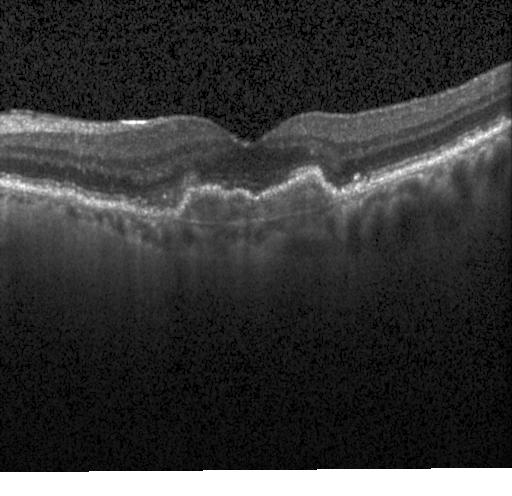 Impression: a choroidal neovascular membrane.